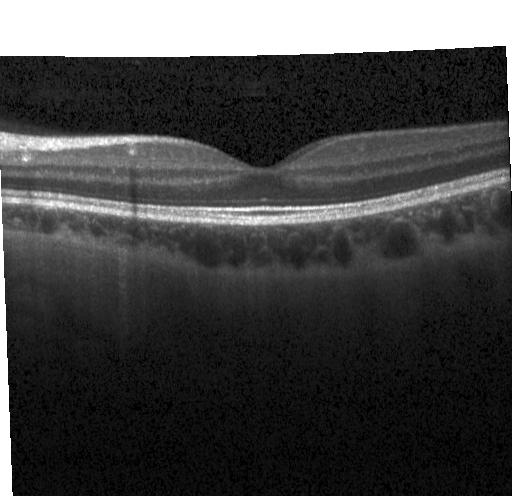 OCT B-scan. Heidelberg Spectralis OCT system.
Dx: no choroidal neovascularization, diabetic macular edema, or drusen.